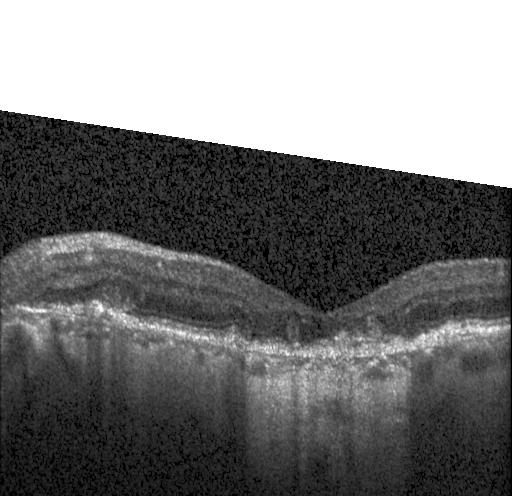 Heidelberg Spectralis · retinal OCT B-scan.
Finding: a choroidal neovascular membrane.